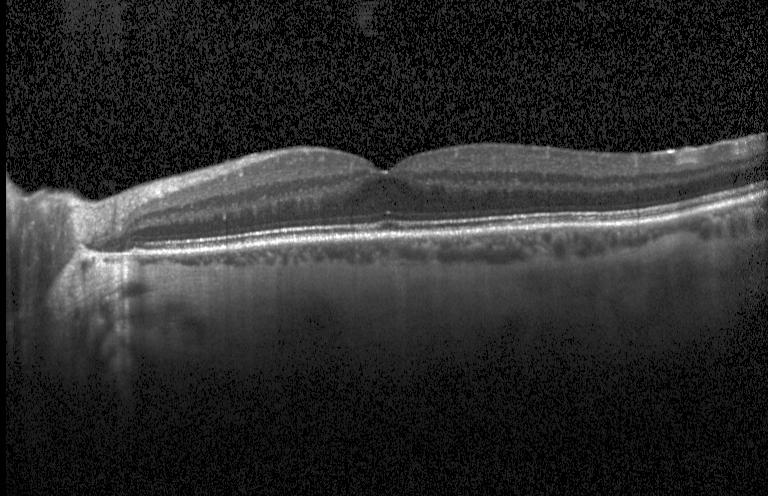

Heidelberg Spectralis OCT system; OCT B-scan; spectral-domain optical coherence tomography; through the macula.
Finding: no choroidal neovascularization, no diabetic macular edema, and no drusen.